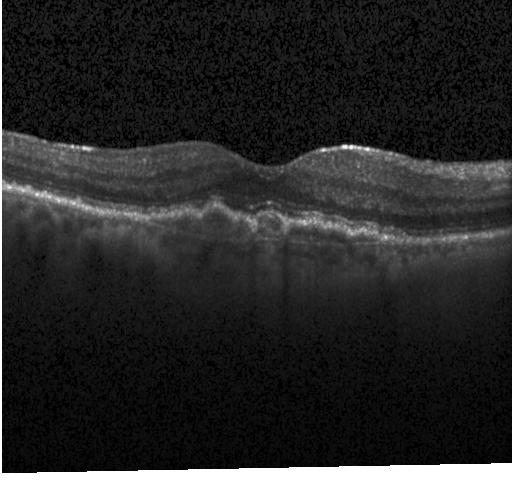 OCT B-scan, Heidelberg Spectralis, spectral-domain optical coherence tomography — Macular OCT: a choroidal neovascular membrane.